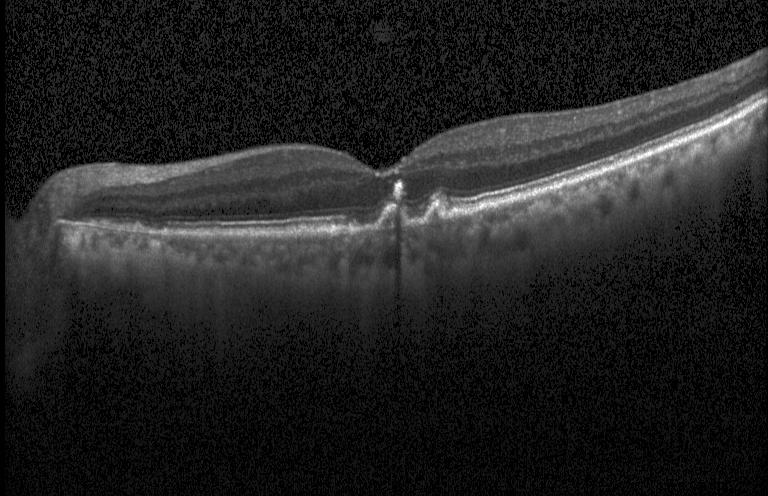

Spectral-domain OCT; optical coherence tomography B-scan
Finding: sub-RPE drusenoid deposits.